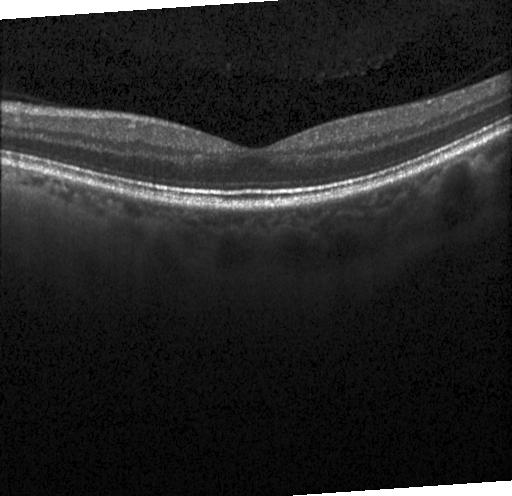 Instrument: Heidelberg Spectralis, optical coherence tomography B-scan, macular scan — The scan shows no CNV, no DME, and no drusen.